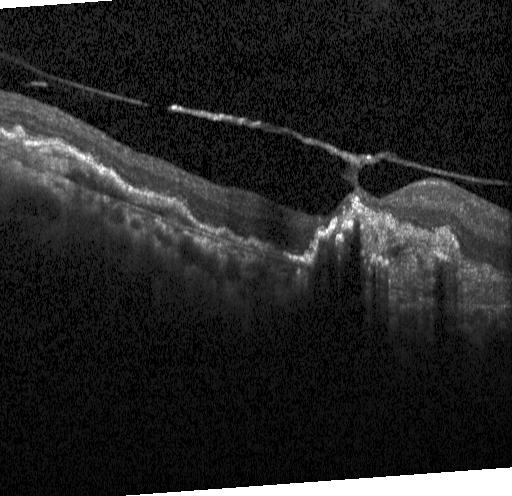 Instrument: Heidelberg Spectralis; fovea-centered; optical coherence tomography scan
Finding: choroidal neovascularization.